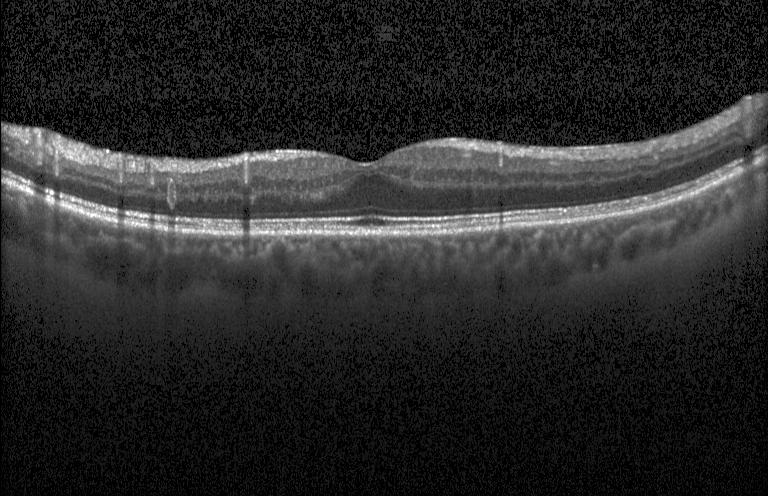 Optical coherence tomography B-scan · SD-OCT.
Finding: no evidence of choroidal neovascularization, diabetic macular edema, or drusen.